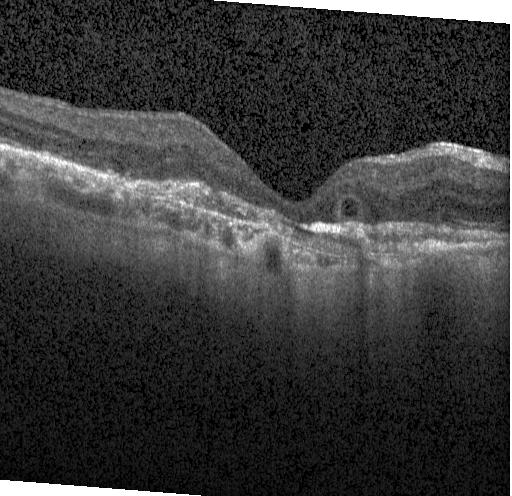 Choroidal neovascularization.